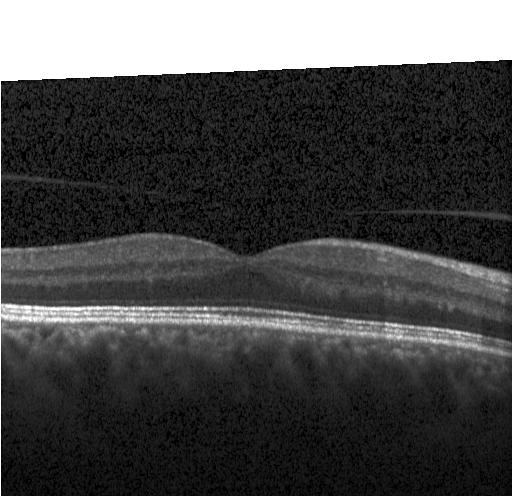 Finding: no CNV, no DME, and no drusen.